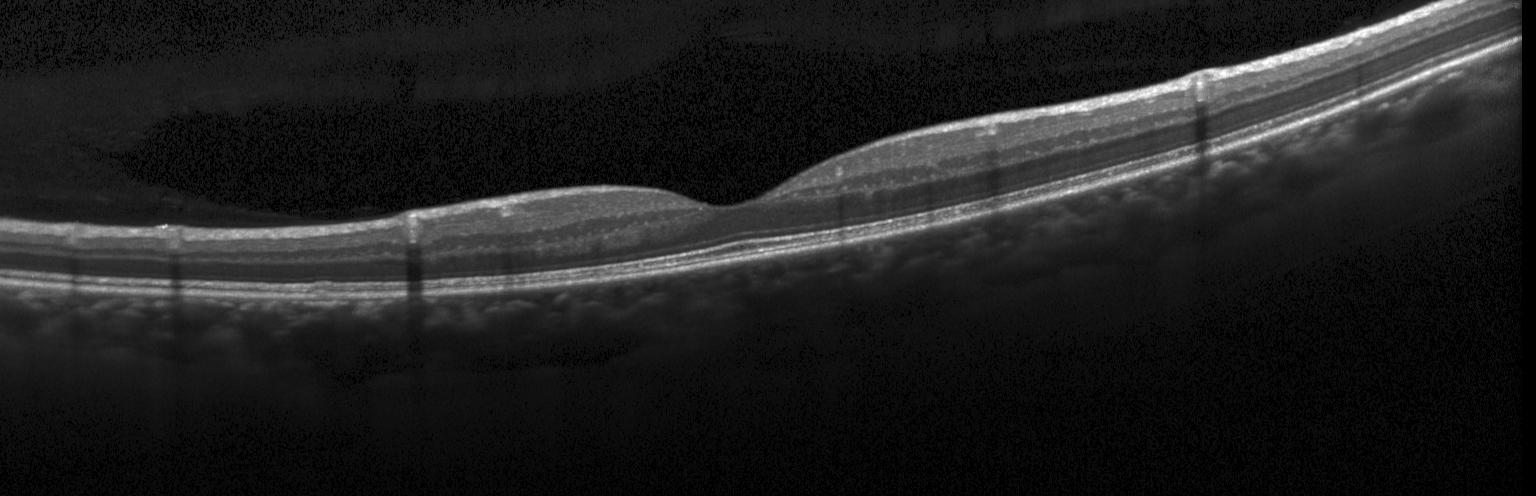 This B-scan demonstrates no evidence of choroidal neovascularization, diabetic macular edema, or drusen.